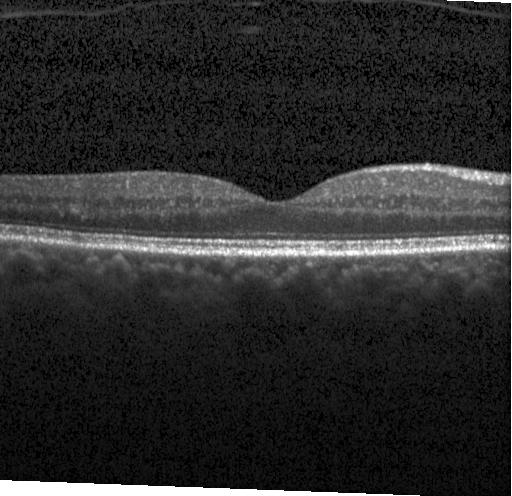 Instrument: Heidelberg Spectralis. Horizontal scan through the fovea. Spectral-domain OCT. OCT line scan.
Impression: no evidence of choroidal neovascularization, diabetic macular edema, or drusen.